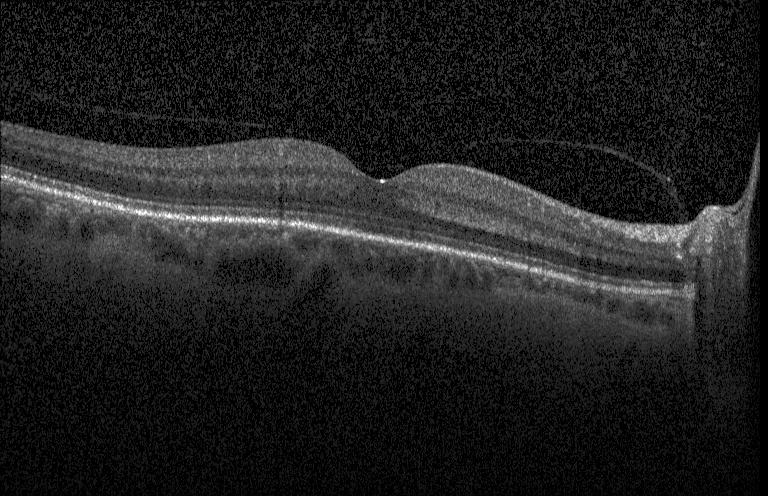
Retinal OCT cross-section — Diagnosis: no CNV, DME, or drusen.